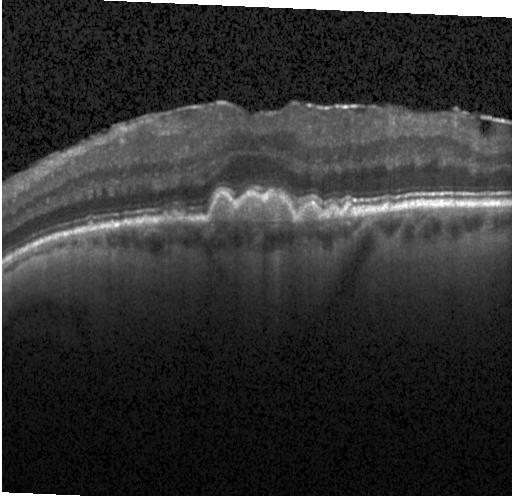

Retinal OCT cross-section, horizontal scan through the fovea, SD-OCT, instrument: Heidelberg Spectralis. Diagnosis: sub-RPE drusenoid deposits.